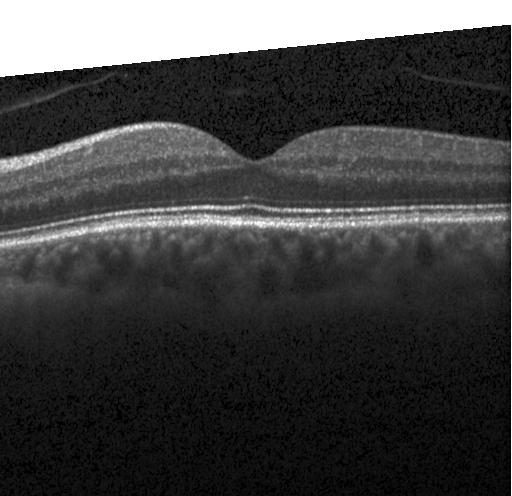
OCT B-scan · spectral-domain OCT · centered on the fovea. The scan shows no choroidal neovascularization, no diabetic macular edema, and no drusen.